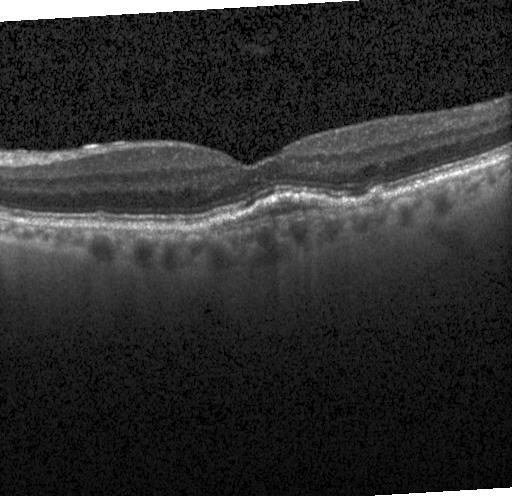 Finding: choroidal neovascularization (CNV).